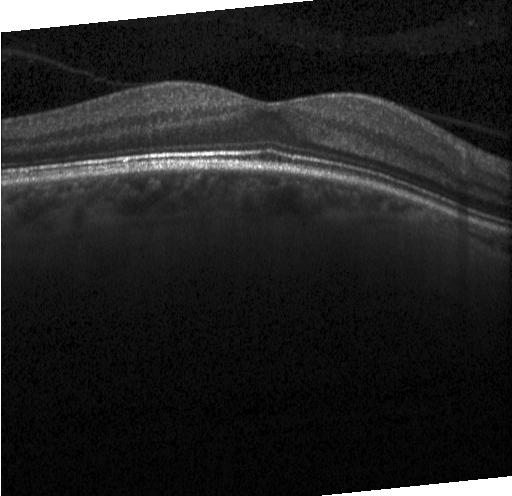 Heidelberg Spectralis · OCT line scan — Assessment: neither choroidal neovascularization, diabetic macular edema, nor drusen.